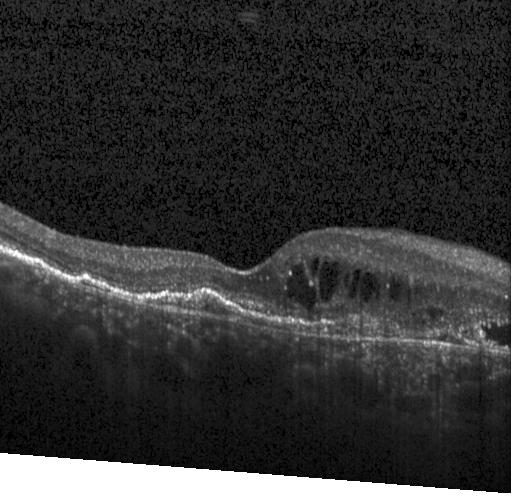

Impression: choroidal neovascularization.